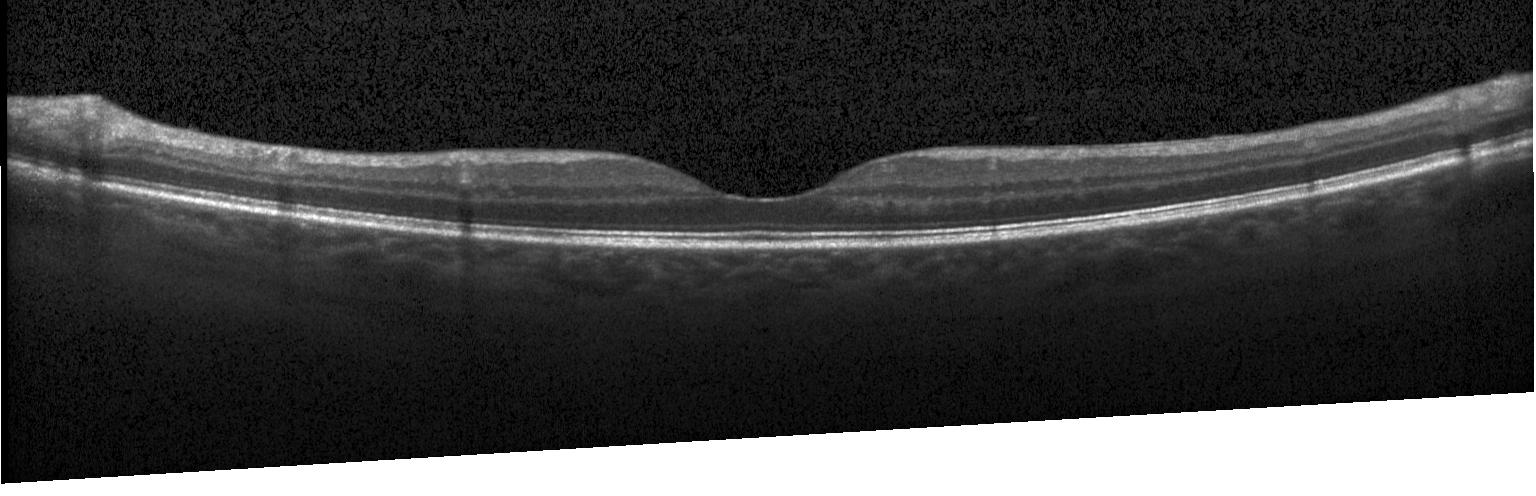 Spectral-domain OCT B-scan: no choroidal neovascularization, no diabetic macular edema, and no drusen.